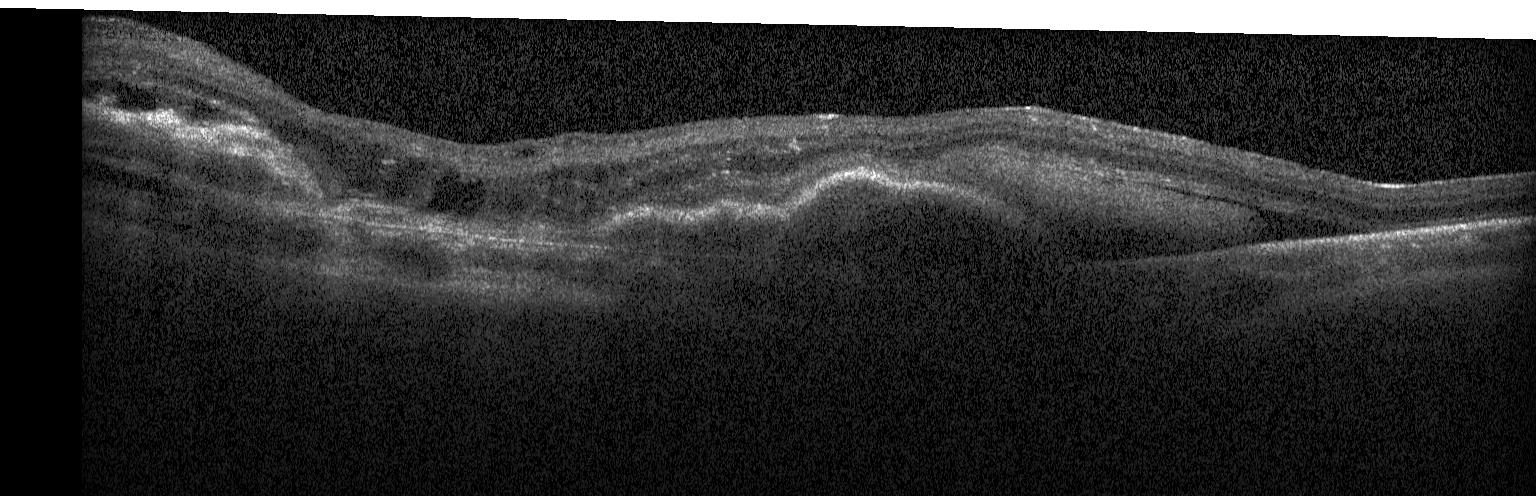
Through the macula. Retinal OCT cross-section
Diagnosis: CNV.